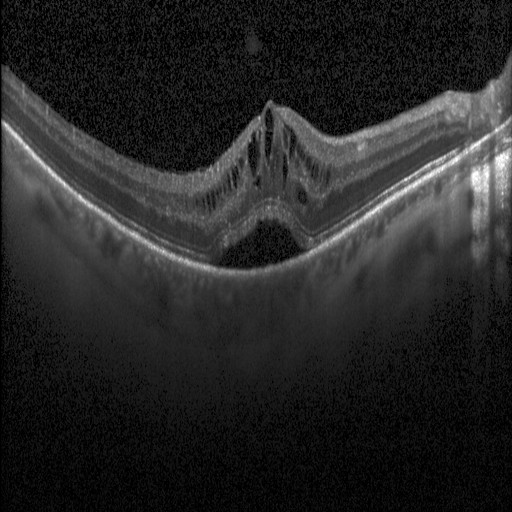
Finding: diabetic macular edema.